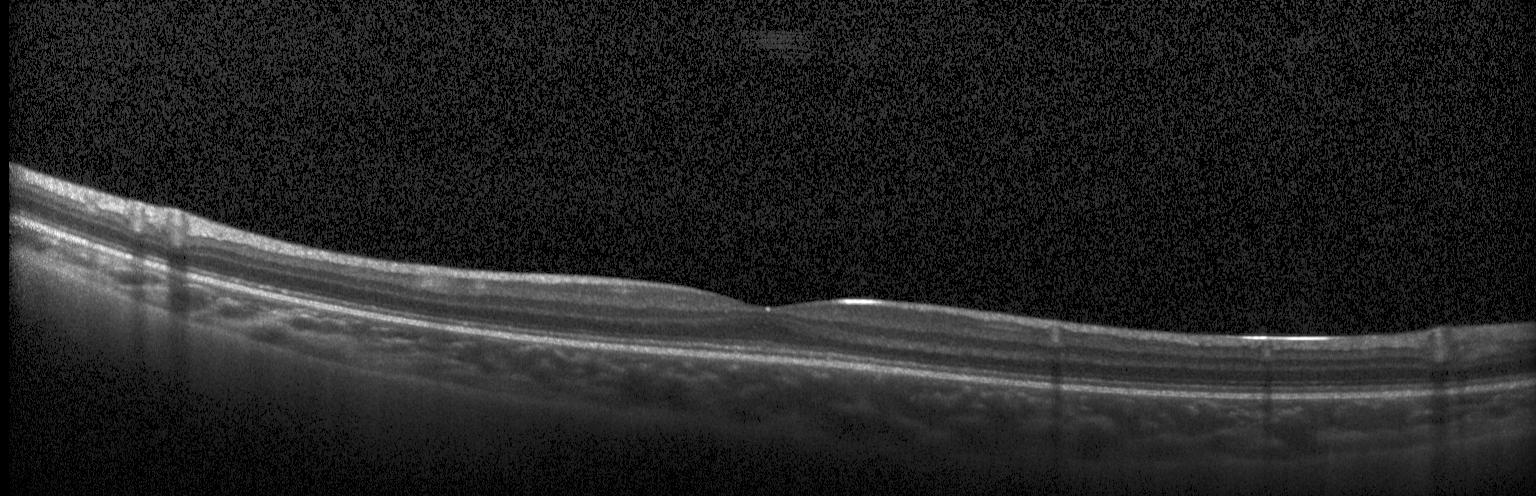

Retinal OCT cross-section showing no evidence of choroidal neovascularization, diabetic macular edema, or drusen.